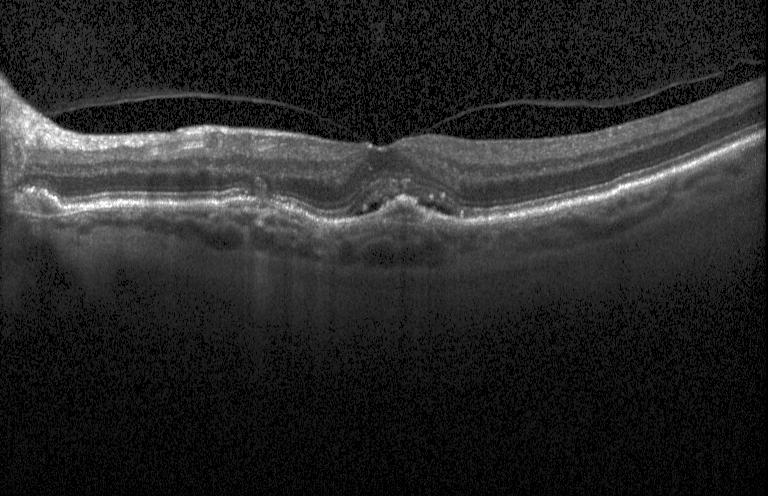
OCT B-scan.
Dx: choroidal neovascularization.